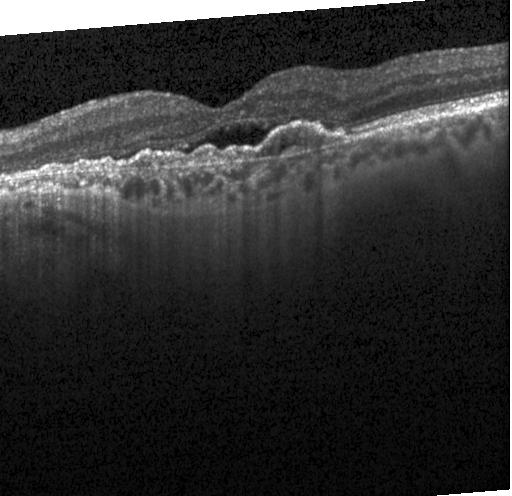 Dx: a choroidal neovascular membrane.